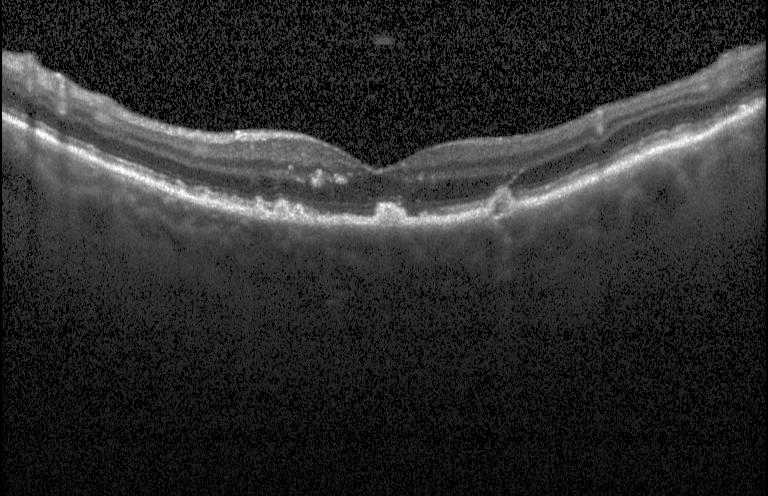

OCT B-scan. A choroidal neovascular membrane.